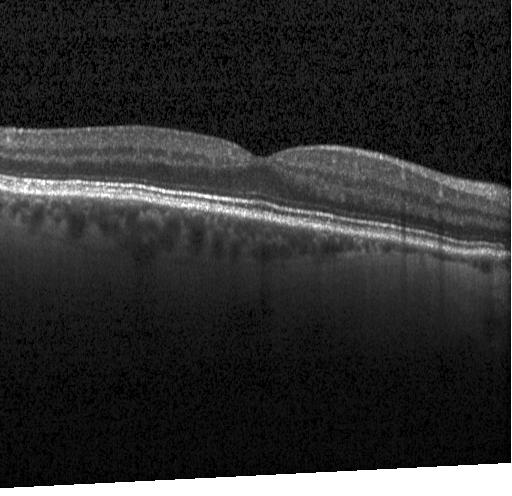
Impression: no CNV, DME, or drusen.